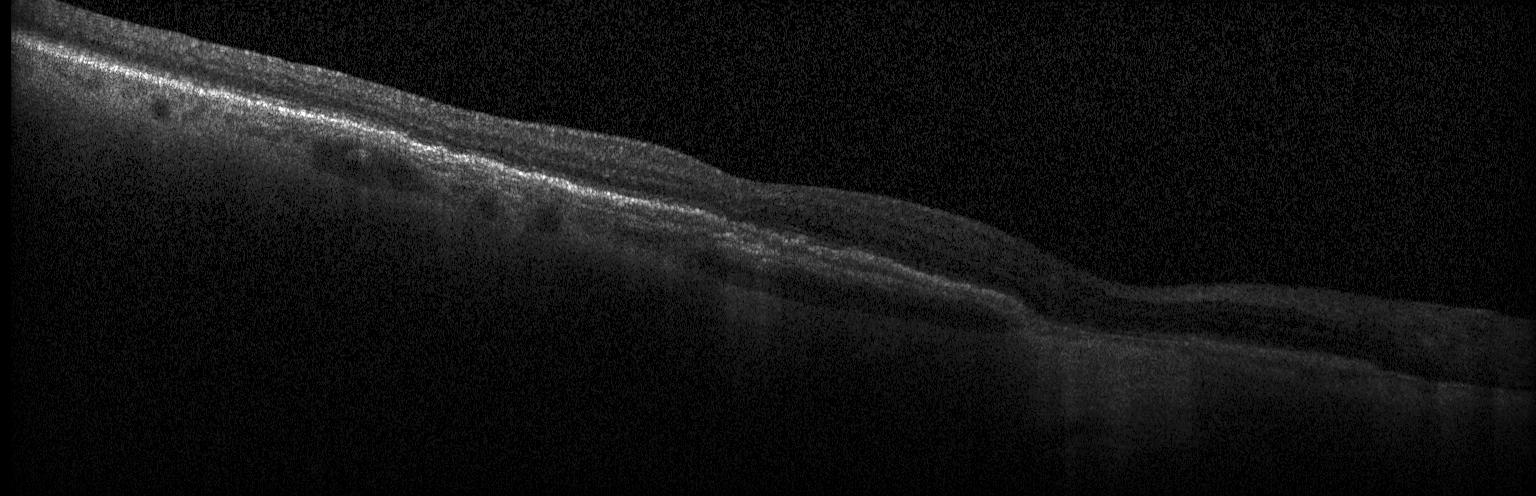
Retinal OCT cross-section — Dx: a choroidal neovascular membrane.